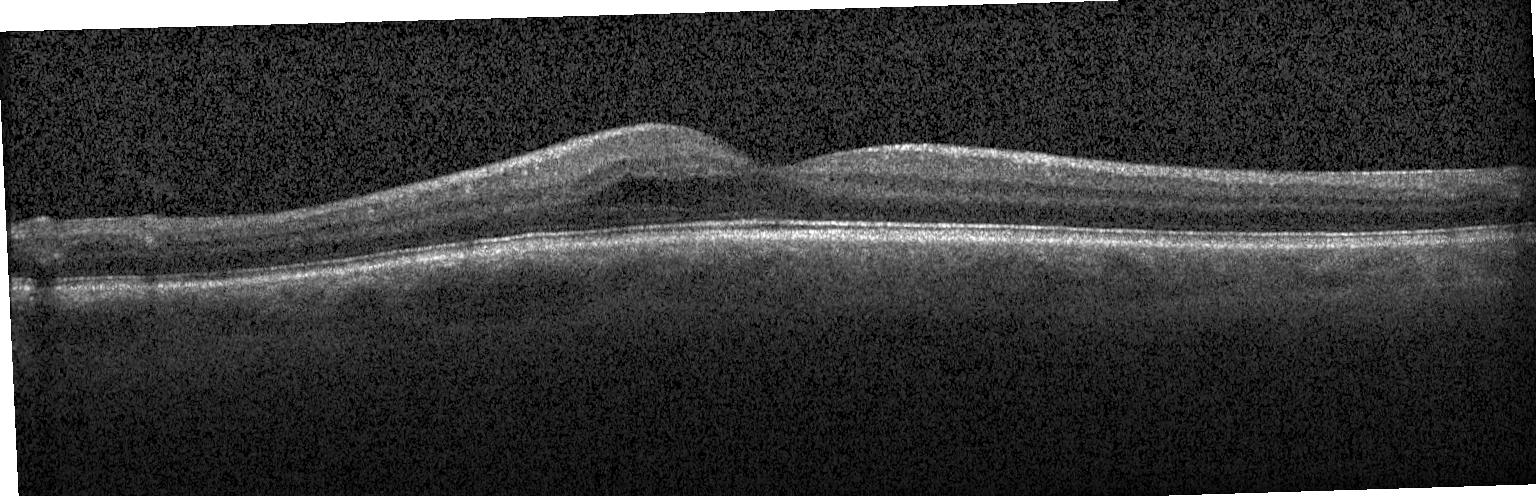

OCT B-scan
This B-scan demonstrates DME.